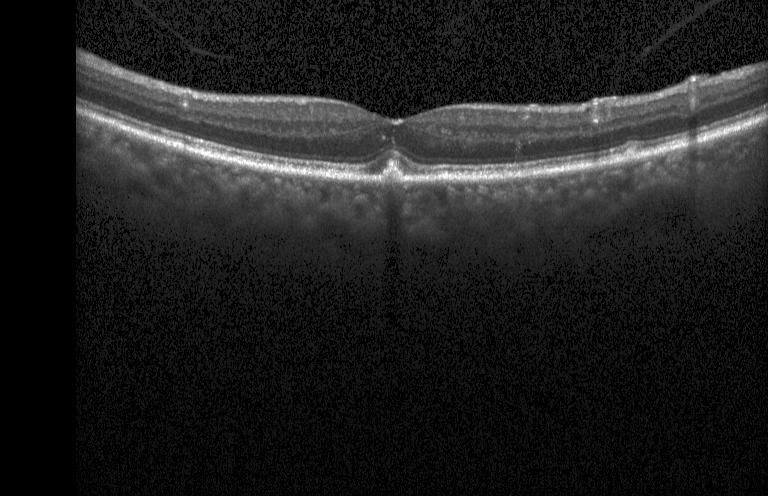
Impression: multiple drusen.